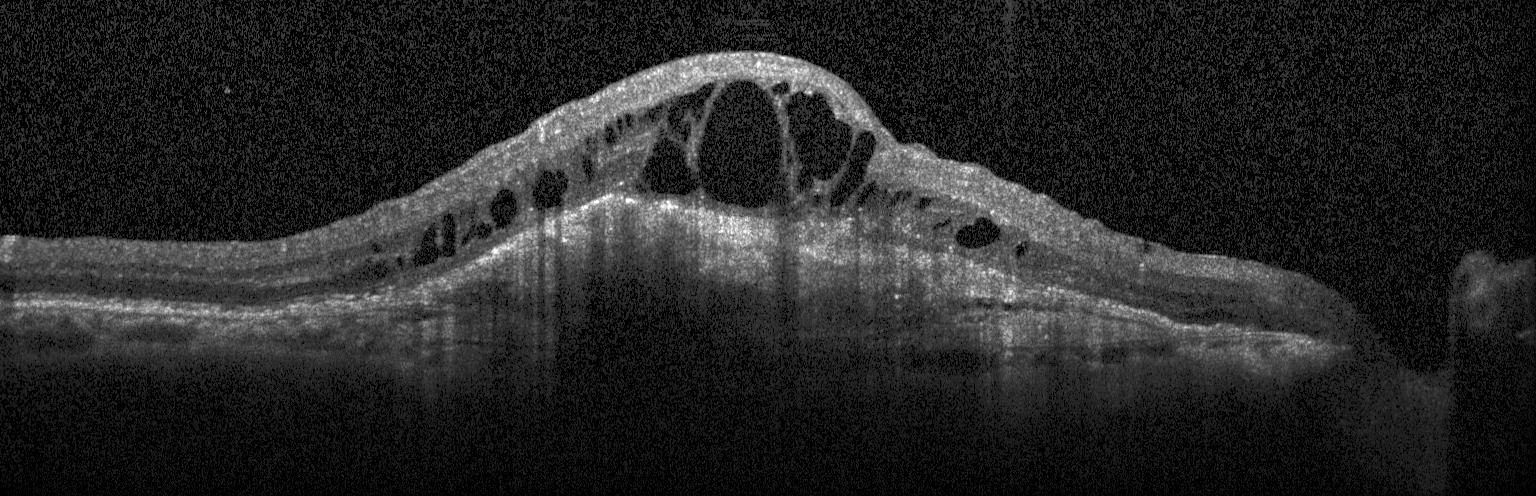 Diagnosis: choroidal neovascularization.